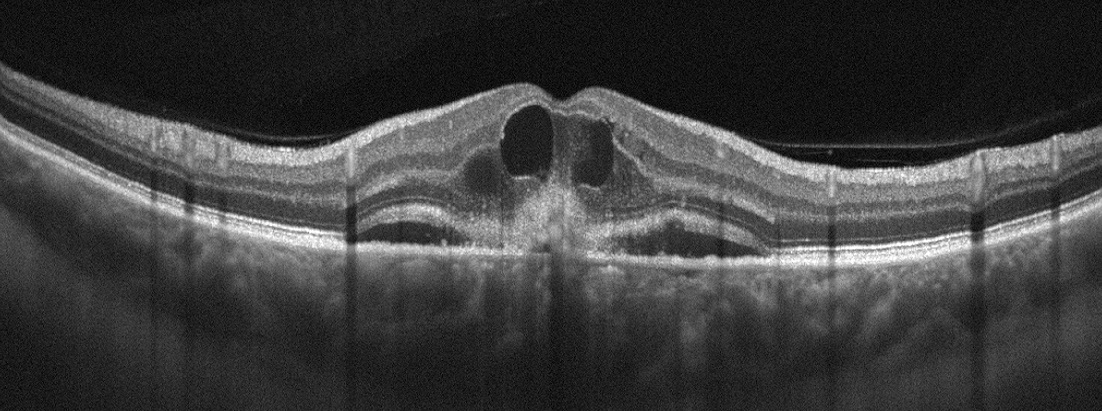 Assessment: AMD.